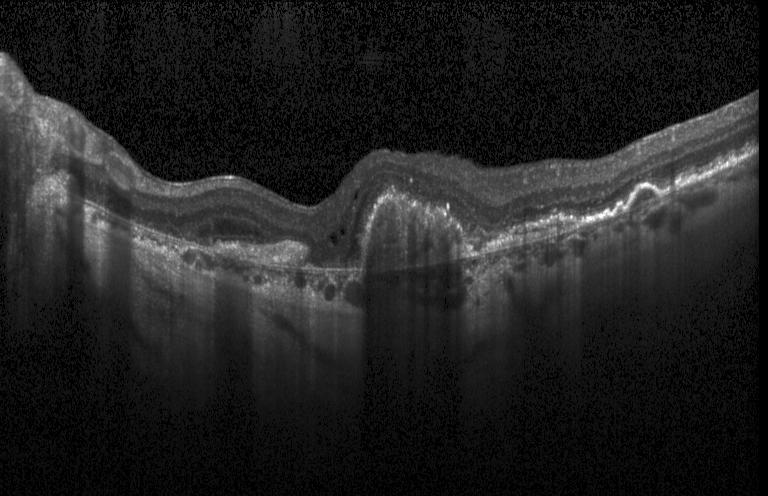 Retinal OCT B-scan; centered on the fovea; Heidelberg Spectralis OCT system; spectral-domain OCT — Impression: a choroidal neovascular membrane.